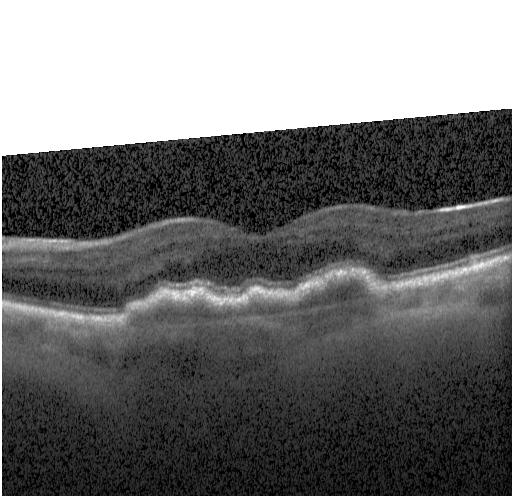

OCT B-scan
Diagnosis: a choroidal neovascular membrane.